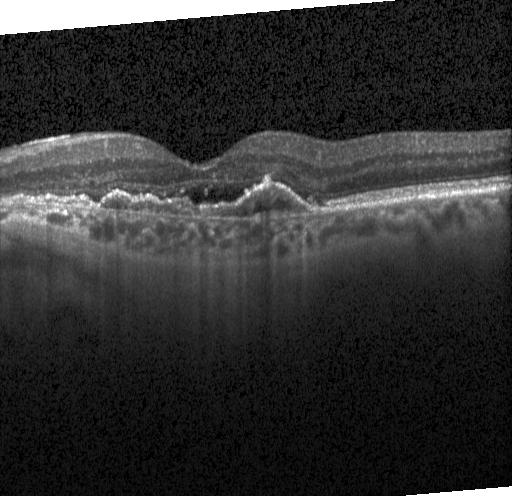
SD-OCT. Retinal OCT B-scan.
Dx: a choroidal neovascular membrane.